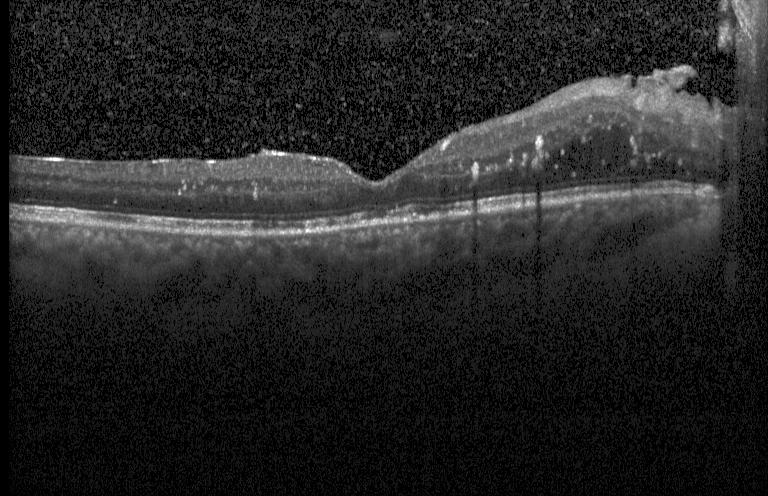 Optical coherence tomography B-scan — Diagnosis: DME.